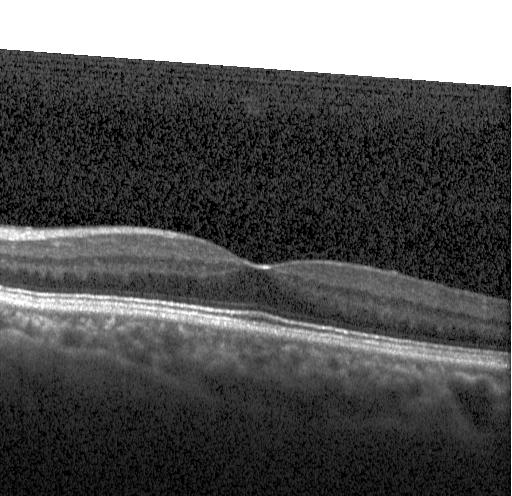

Retinal OCT cross-section
Assessment: no choroidal neovascularization, no diabetic macular edema, and no drusen.